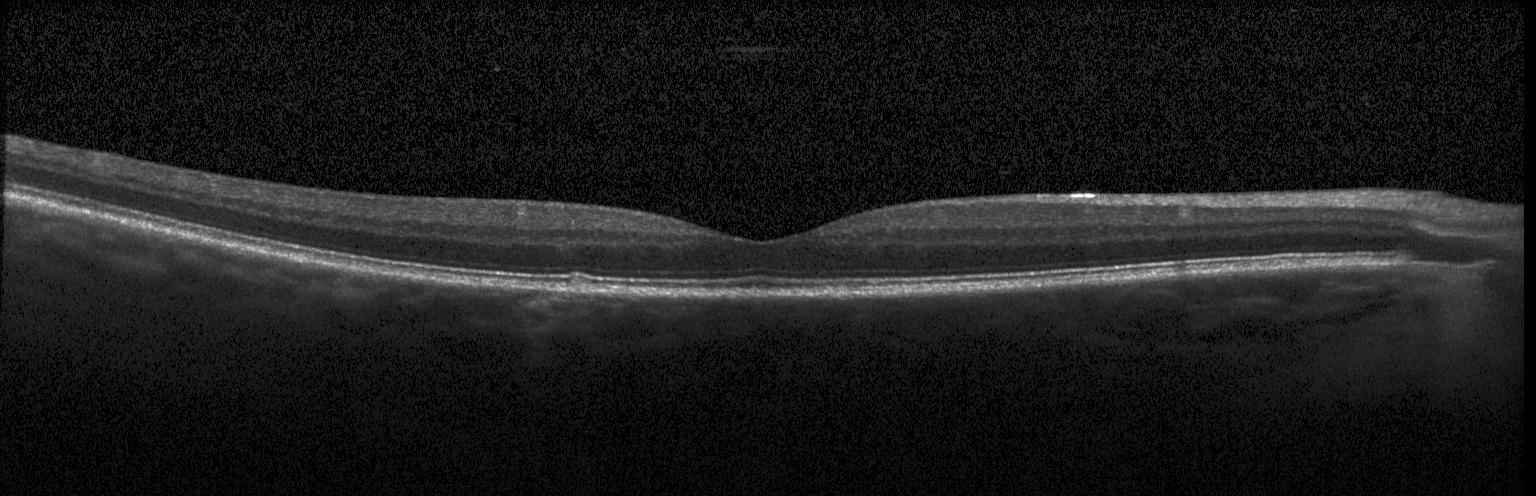 Impression: no evidence of CNV, DME, or drusen.